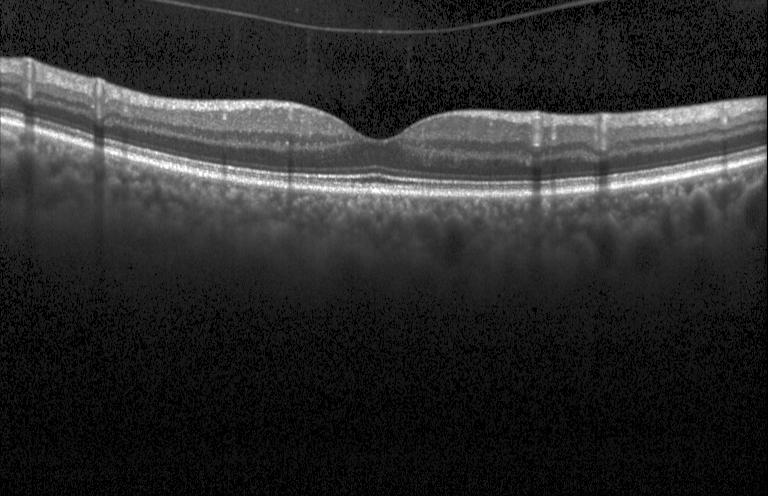 OCT B-scan, macular scan.
Impression: neither choroidal neovascularization, diabetic macular edema, nor drusen.